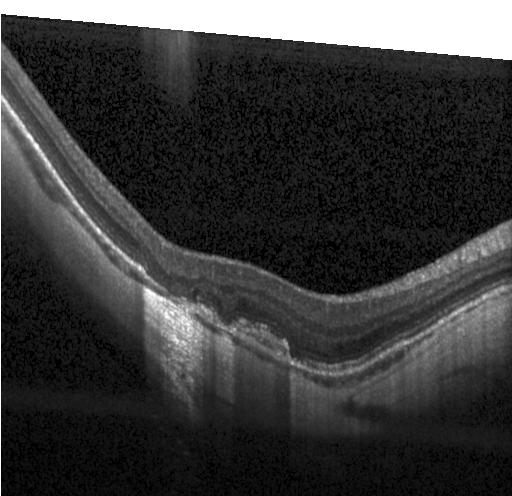
Instrument: Heidelberg Spectralis; through the macula; OCT B-scan; SD-OCT — Diagnosis: a choroidal neovascular membrane.